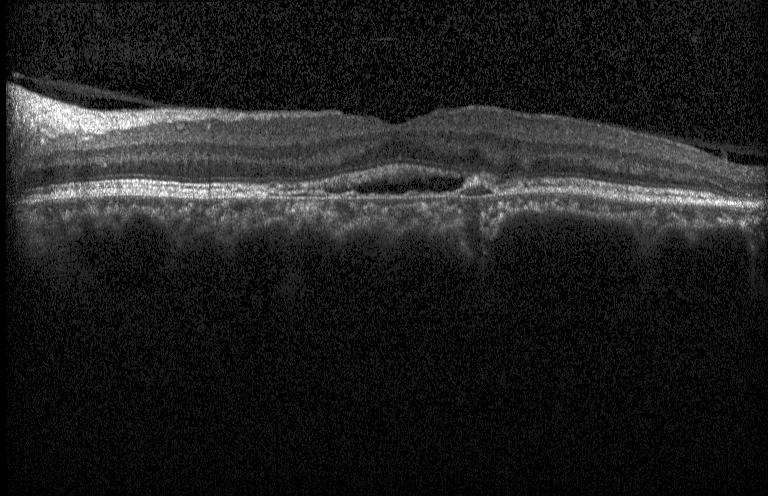 Spectral-domain optical coherence tomography, optical coherence tomography scan, through the macula. Diagnosis: a choroidal neovascular membrane.